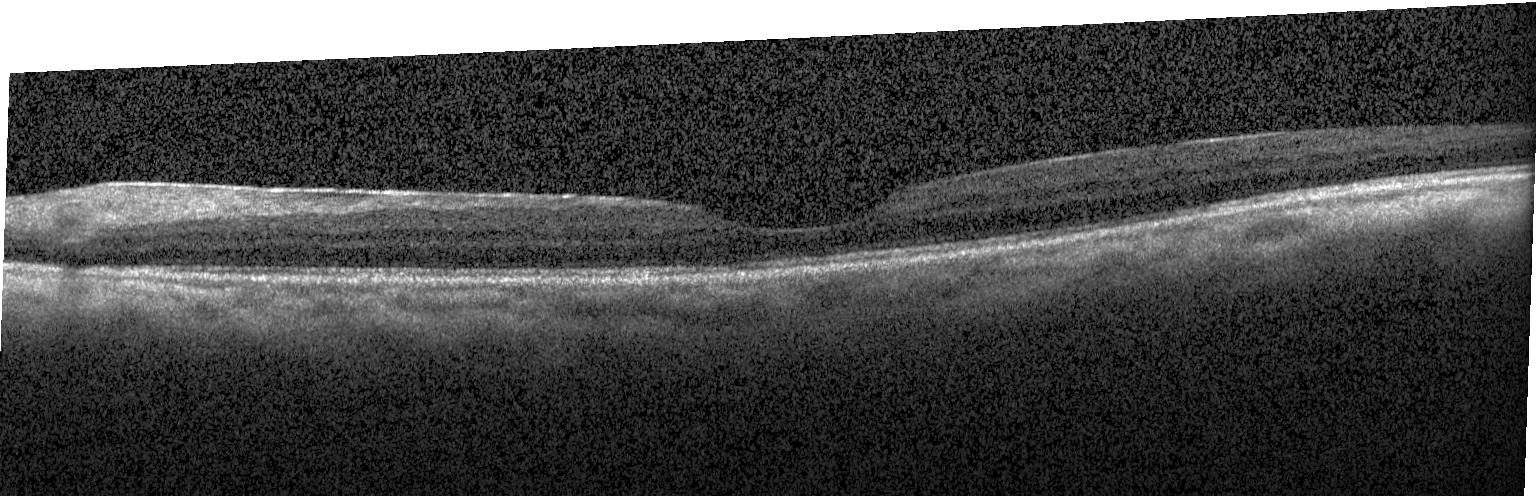 Retinal OCT B-scan — Dx: no CNV, no DME, and no drusen.